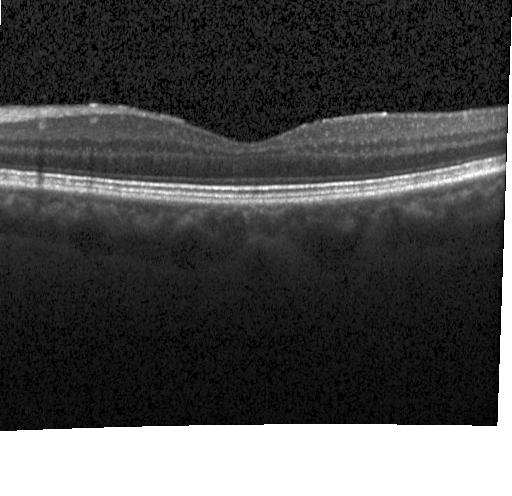
Spectral-domain OCT; instrument: Heidelberg Spectralis; centered on the fovea; optical coherence tomography scan. Finding: no evidence of choroidal neovascularization, diabetic macular edema, or drusen.